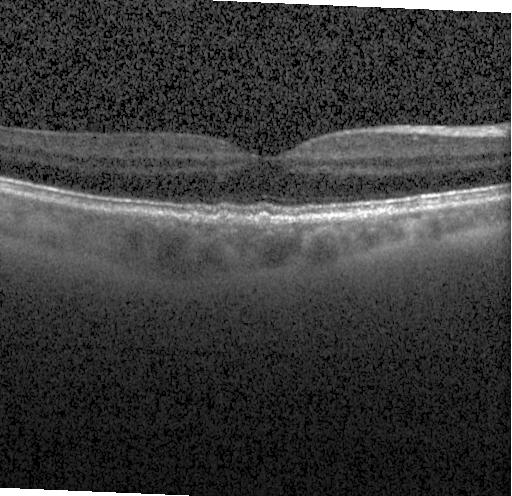

Sub-RPE drusenoid deposits.